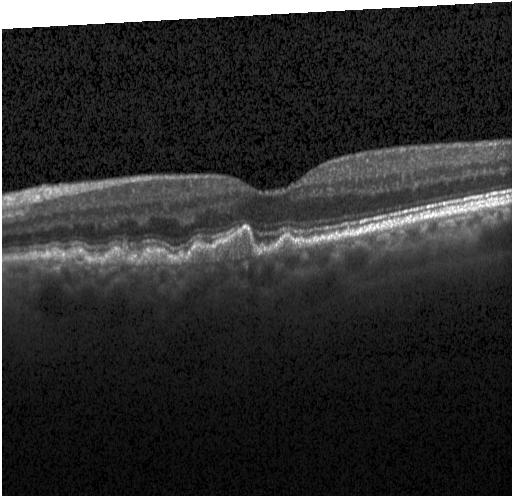
Heidelberg Spectralis OCT system. Fovea-centered. SD-OCT. Optical coherence tomography scan.
Drusen.